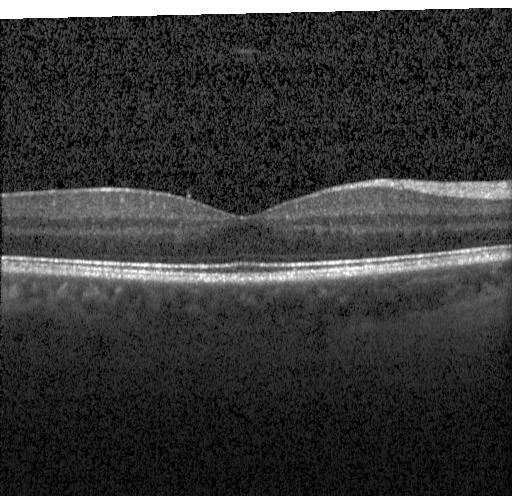
Retinal OCT B-scan, centered on the fovea, spectral-domain optical coherence tomography, instrument: Heidelberg Spectralis — Dx: neither CNV, DME, nor drusen.